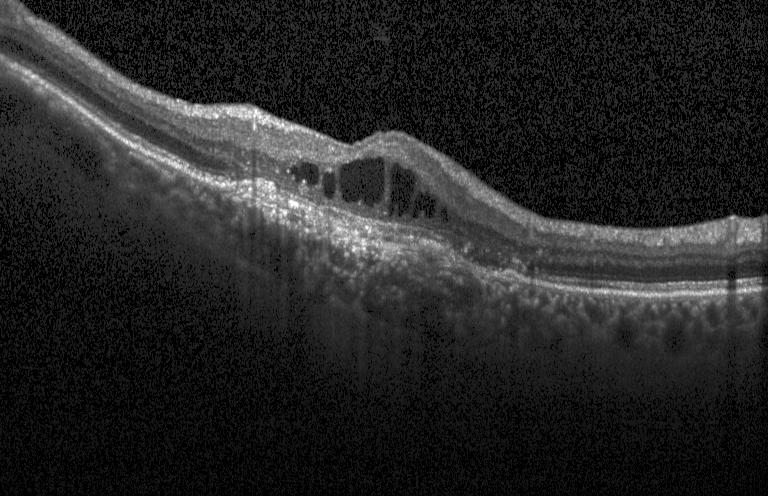 Heidelberg Spectralis · retinal OCT B-scan. The scan shows choroidal neovascularization.